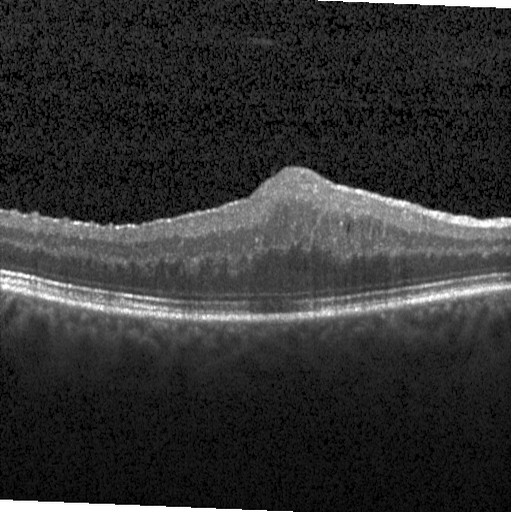 Instrument: Heidelberg Spectralis. OCT B-scan. SD-OCT. Centered on the fovea. Diagnosis: diabetic macular edema (DME).